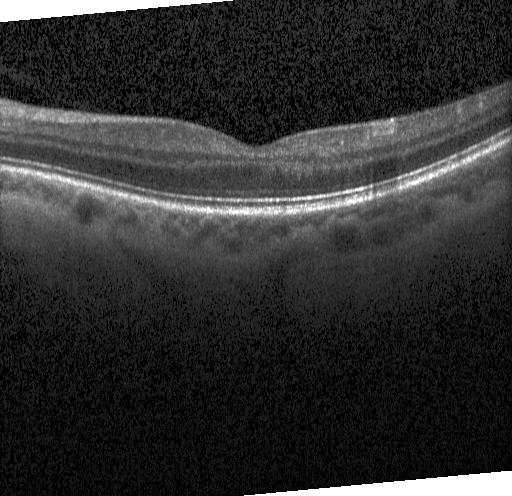 Retinal OCT B-scan. Assessment: no evidence of choroidal neovascularization, diabetic macular edema, or drusen.